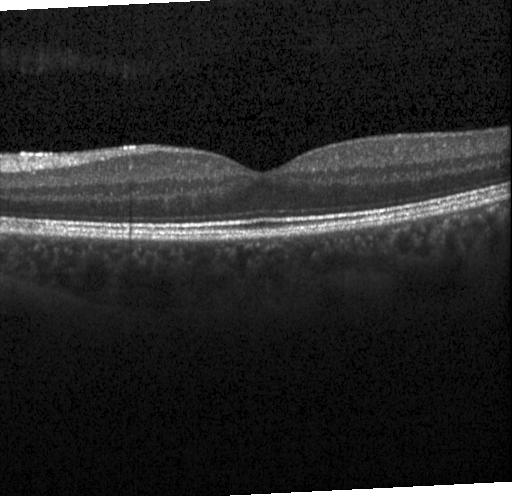 Retinal OCT cross-section
Impression: no CNV, DME, or drusen.